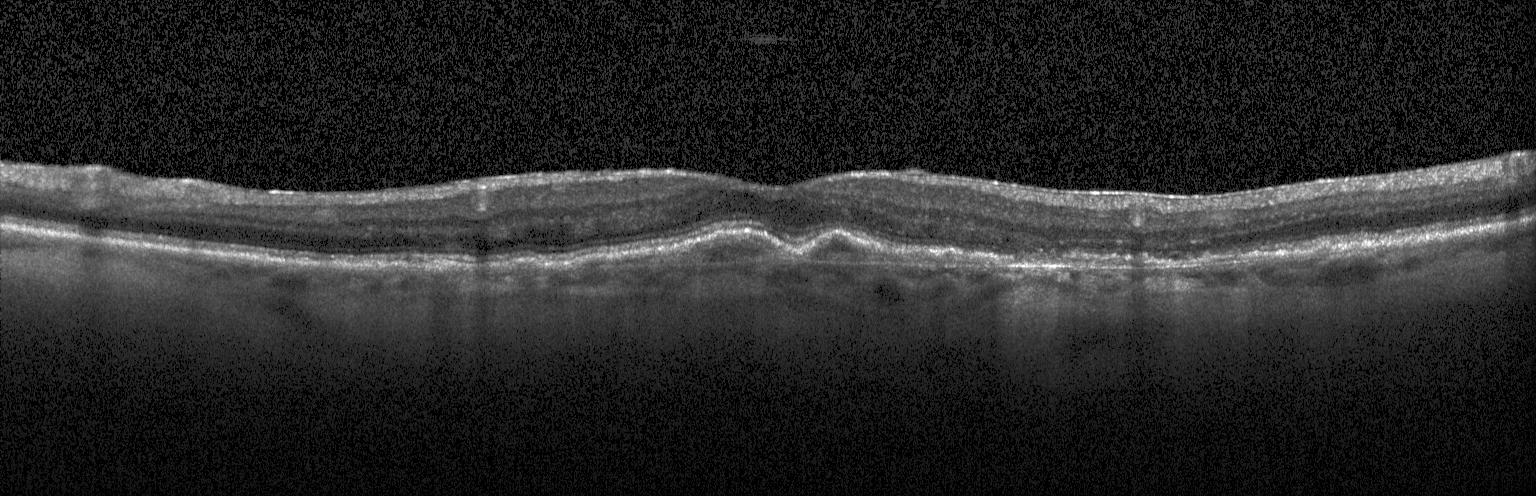
Retinal OCT B-scan. Spectral-domain optical coherence tomography. OCT finding: choroidal neovascularization (CNV).